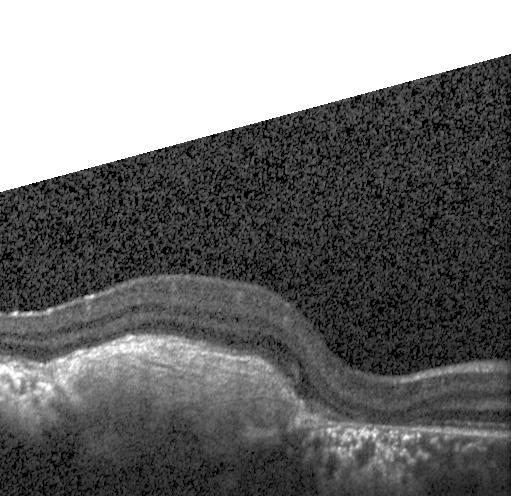 Retinal OCT cross-section. Centered on the fovea — Finding: choroidal neovascularization.